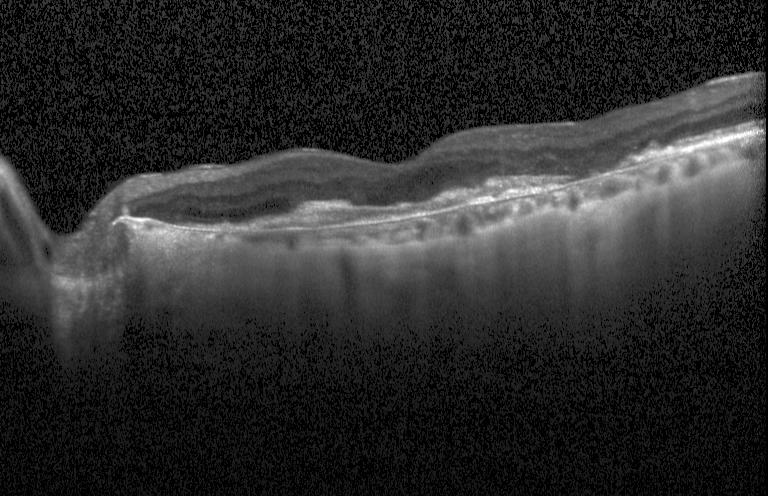 Spectral-domain OCT. Retinal OCT cross-section. Centered on the fovea. Acquired on a Heidelberg Spectralis. Impression: choroidal neovascularization (CNV).